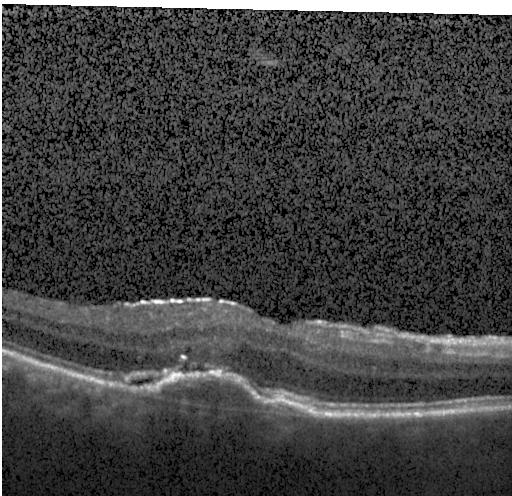 Spectral-domain optical coherence tomography, retinal OCT cross-section, through the macula, Heidelberg Spectralis OCT system — Finding: choroidal neovascularization.